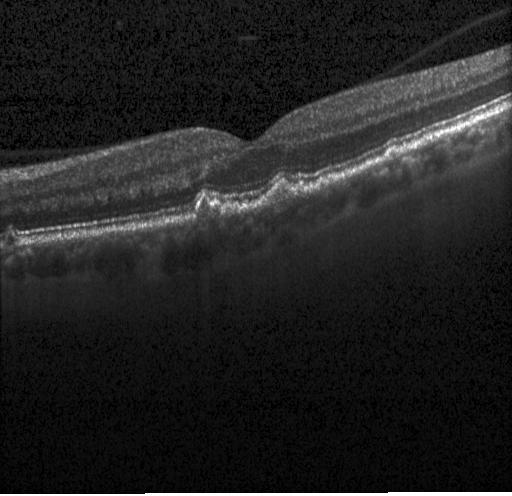

Dx: drusen.